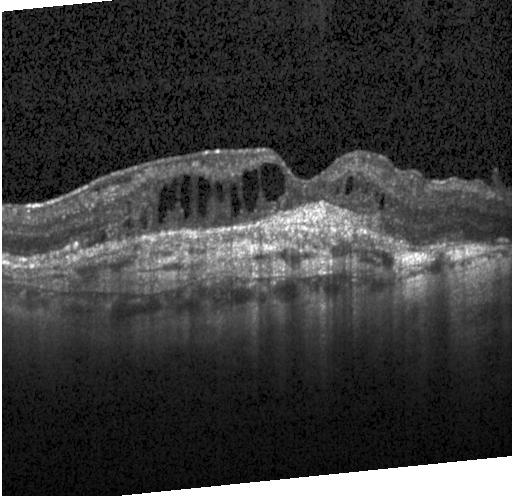

Retinal OCT cross-section showing a choroidal neovascular membrane.